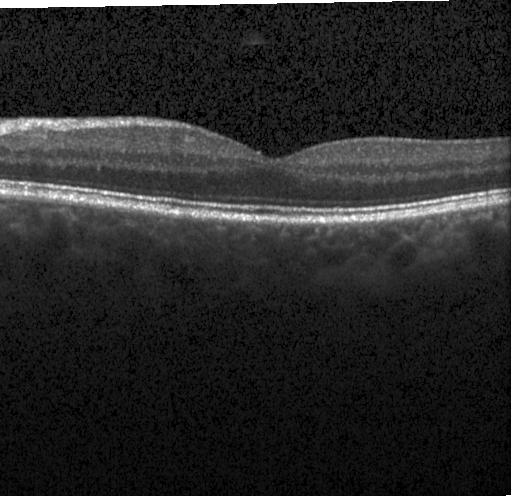 Optical coherence tomography scan
This B-scan demonstrates neither choroidal neovascularization, diabetic macular edema, nor drusen.